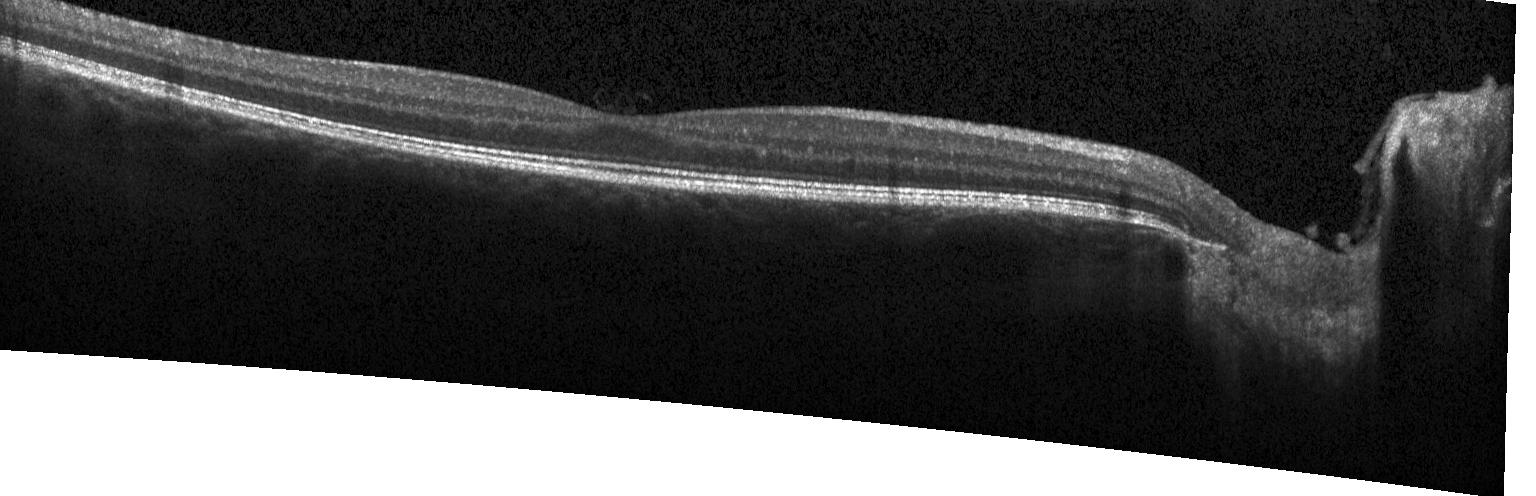 Fovea-centered; retinal OCT cross-section; instrument: Heidelberg Spectralis
Impression: no evidence of CNV, DME, or drusen.